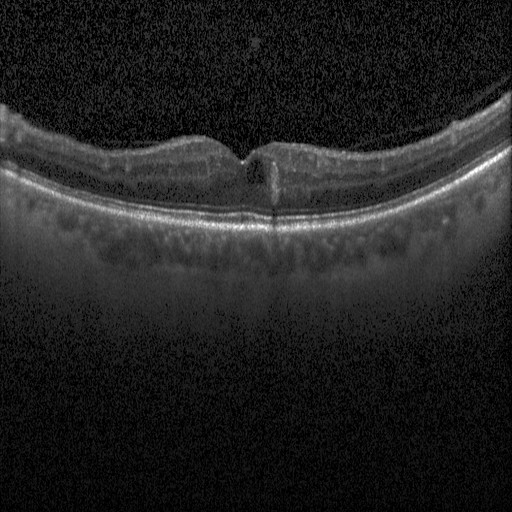

Heidelberg Spectralis OCT system; OCT line scan; spectral-domain optical coherence tomography. This B-scan demonstrates diabetic macular edema.